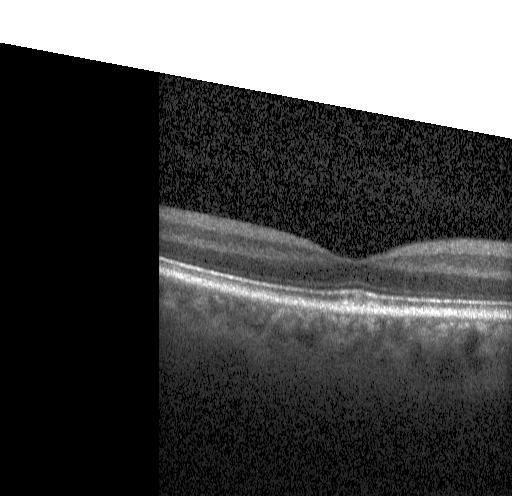

OCT line scan — Dx: no CNV, no DME, and no drusen.